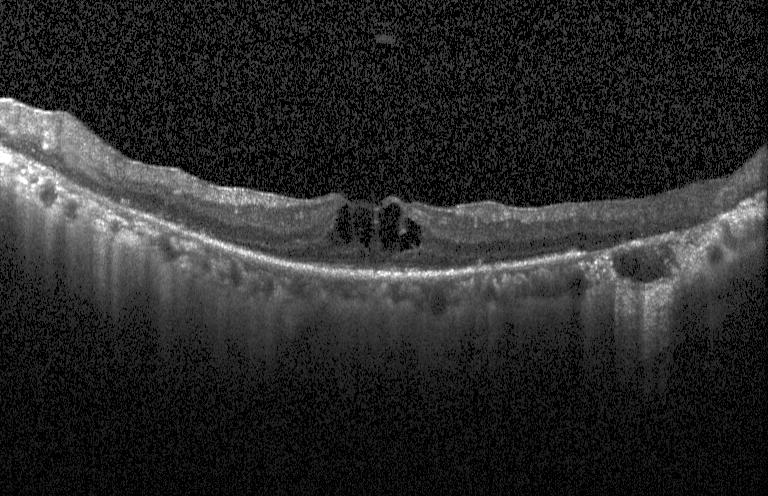
Instrument: Heidelberg Spectralis, through the macula, optical coherence tomography B-scan, SD-OCT.
This B-scan demonstrates diabetic macular edema (DME).